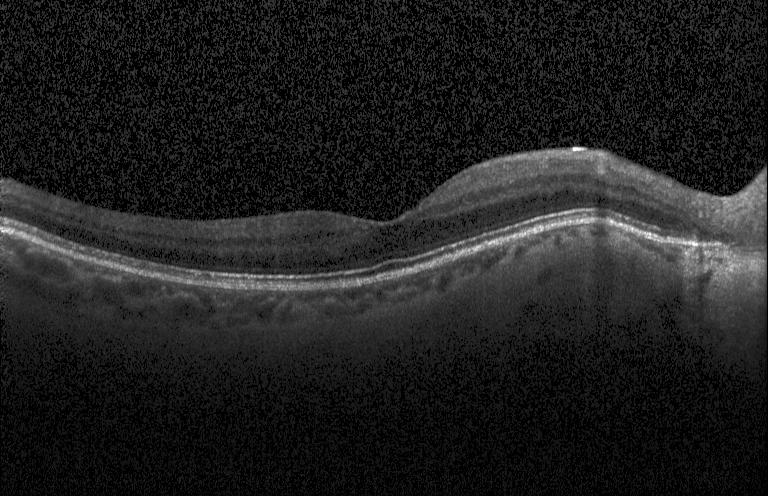 No choroidal neovascularization, no diabetic macular edema, and no drusen.